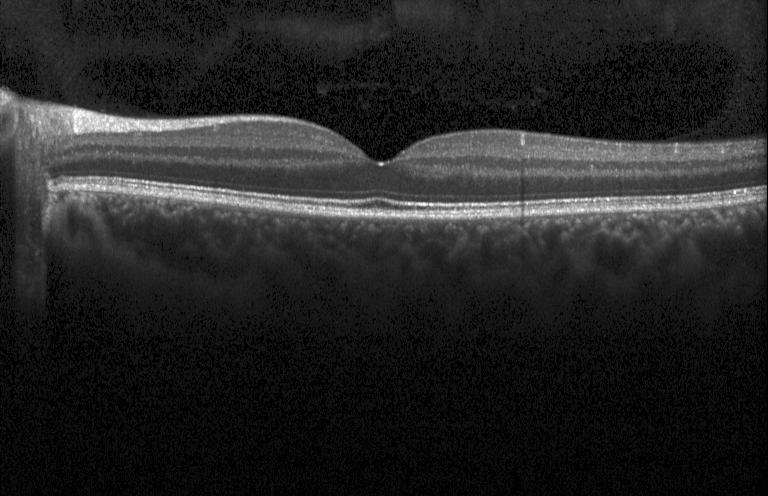
Impression: neither choroidal neovascularization, diabetic macular edema, nor drusen.